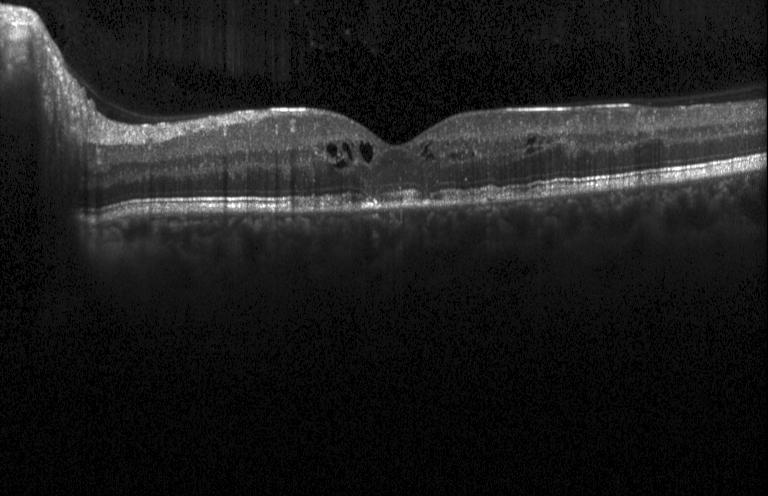

OCT scan showing DME.